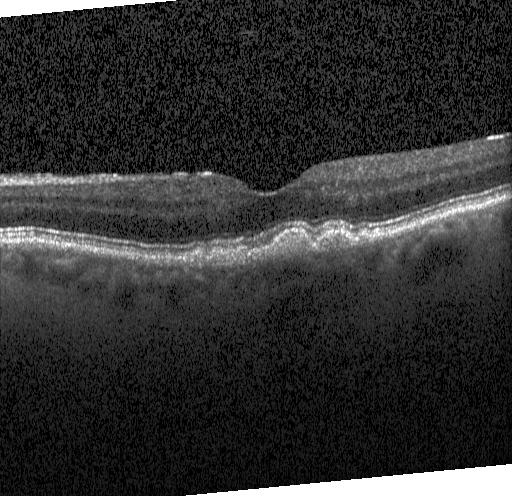 Retinal OCT cross-section.
Assessment: sub-RPE drusenoid deposits.